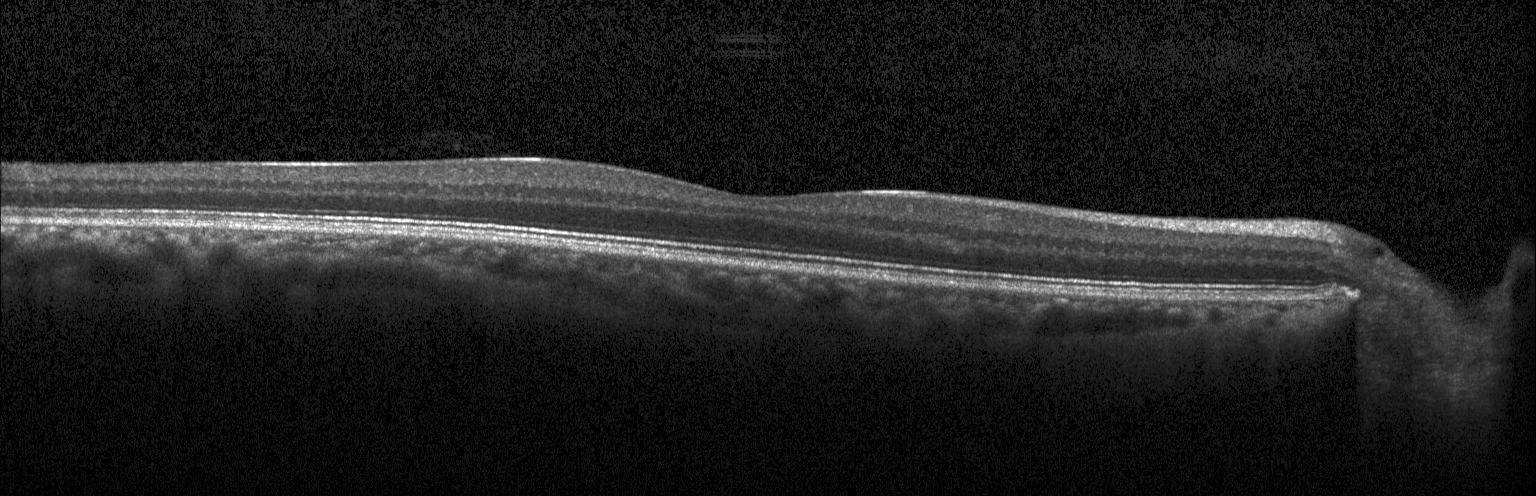 Fovea-centered · spectral-domain optical coherence tomography · Heidelberg Spectralis OCT system · retinal OCT cross-section. The scan shows no choroidal neovascularization, no diabetic macular edema, and no drusen.